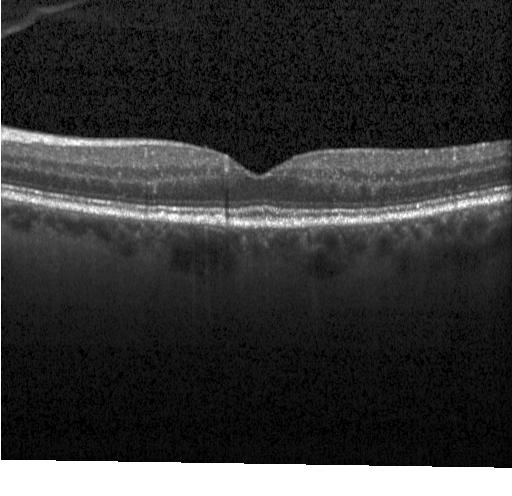

Diagnosis: no choroidal neovascularization, no diabetic macular edema, and no drusen.